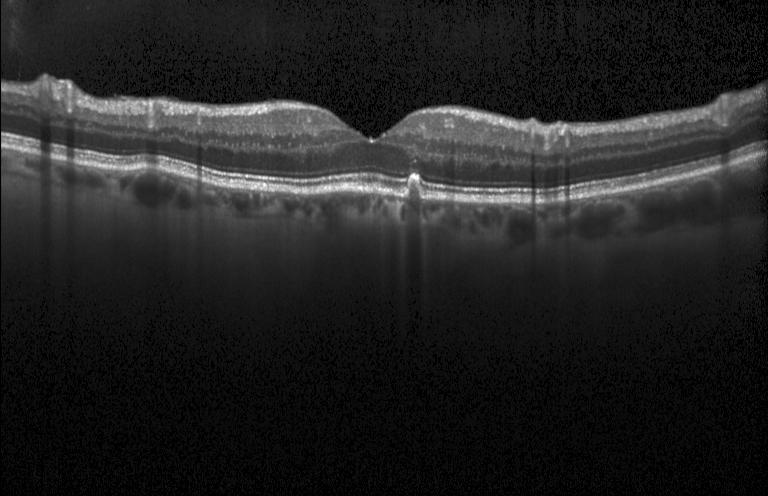 Diagnosis: multiple drusen.